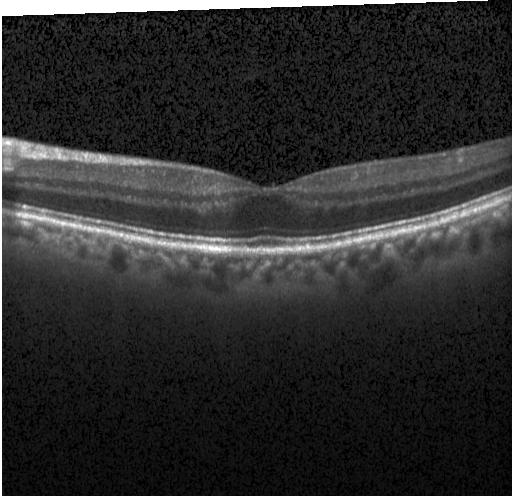

Macular OCT: no evidence of CNV, DME, or drusen.